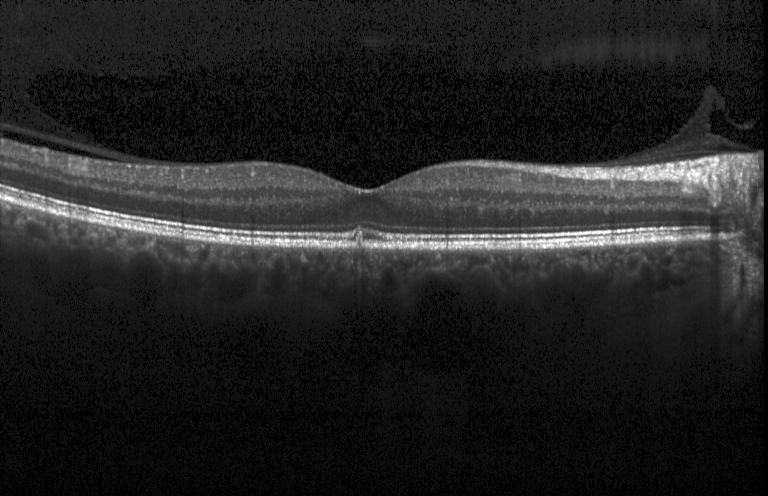 Optical coherence tomography scan.
Sub-RPE drusenoid deposits.